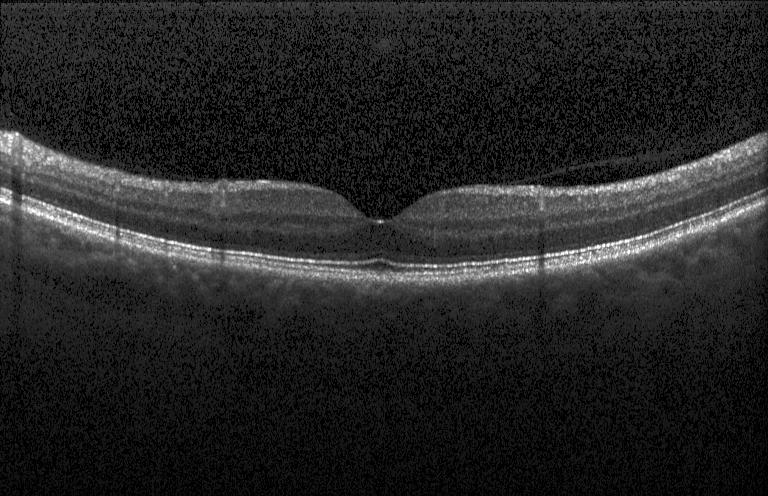 Dx: neither choroidal neovascularization, diabetic macular edema, nor drusen.